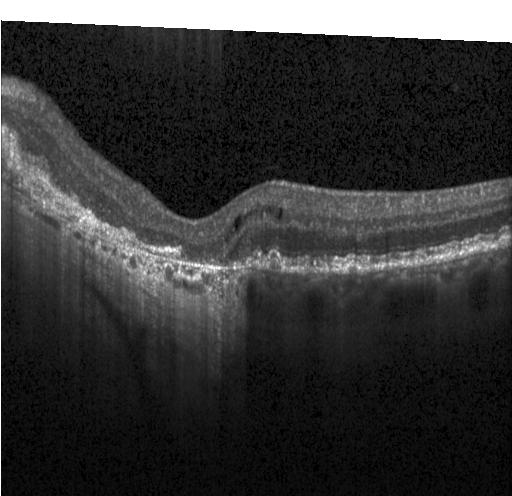
Retinal OCT B-scan; spectral-domain optical coherence tomography; horizontal scan through the fovea — Impression: CNV.